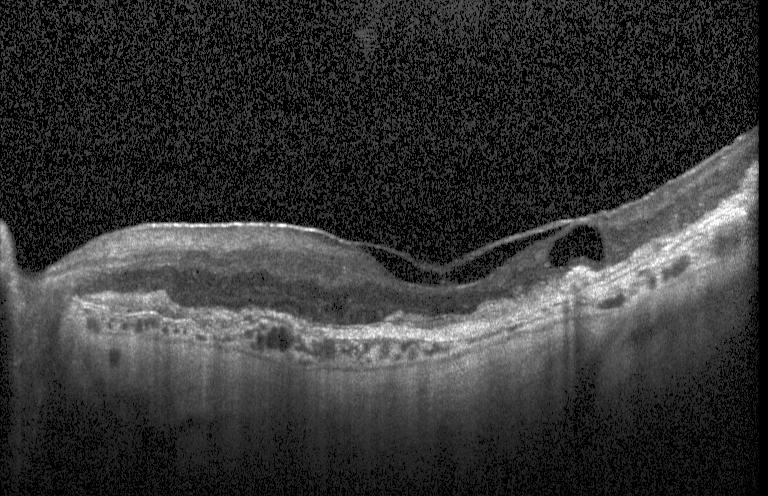 Dx: a choroidal neovascular membrane.